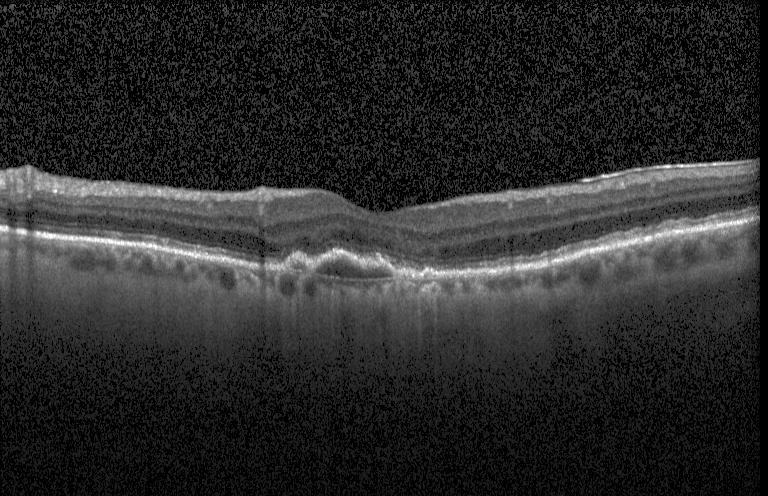

Diagnosis: CNV.